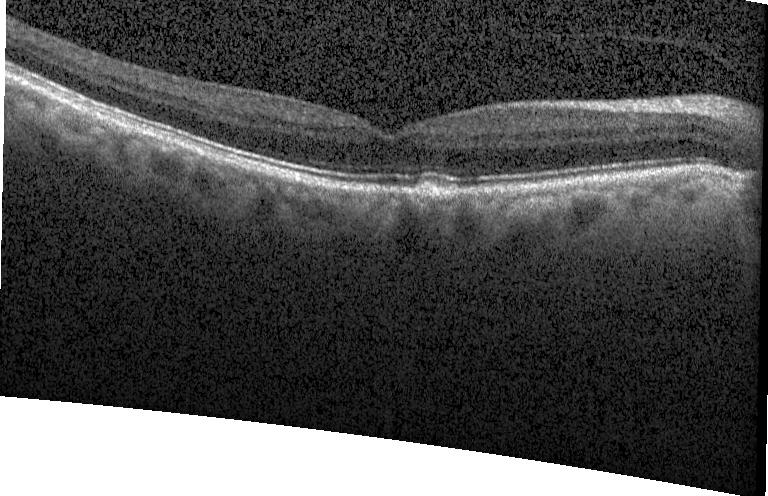

Optical coherence tomography scan. Diagnosis: sub-RPE drusenoid deposits.